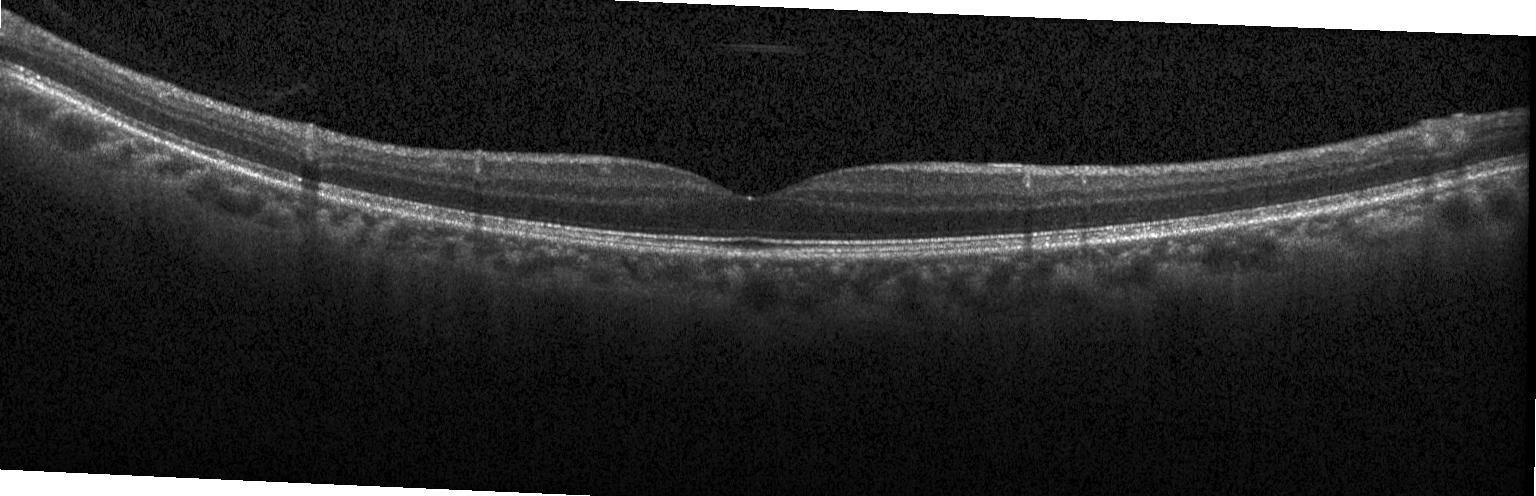

Spectral-domain OCT B-scan: no CNV, DME, or drusen.